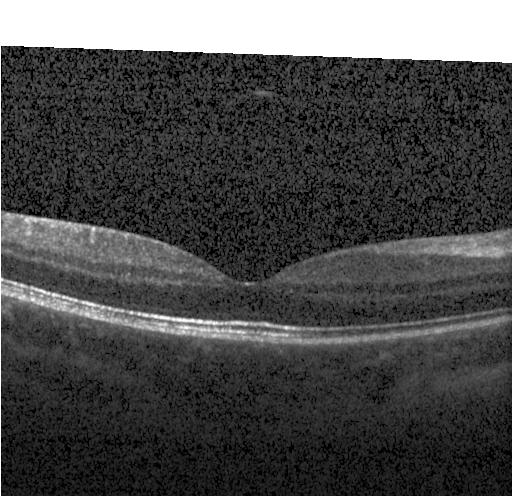

OCT finding: no evidence of choroidal neovascularization, diabetic macular edema, or drusen.